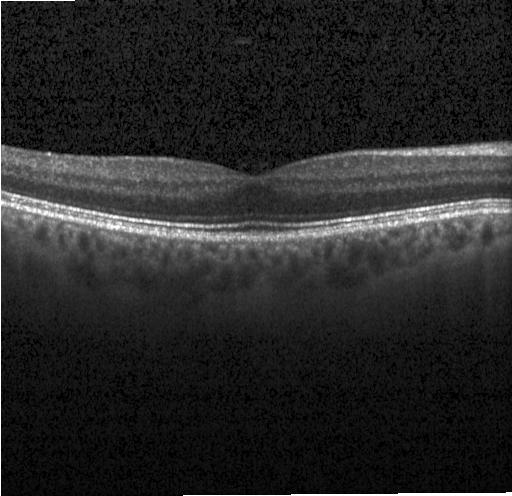 Through the macula · retinal OCT B-scan · SD-OCT · acquired on a Heidelberg Spectralis
The scan shows neither CNV, DME, nor drusen.